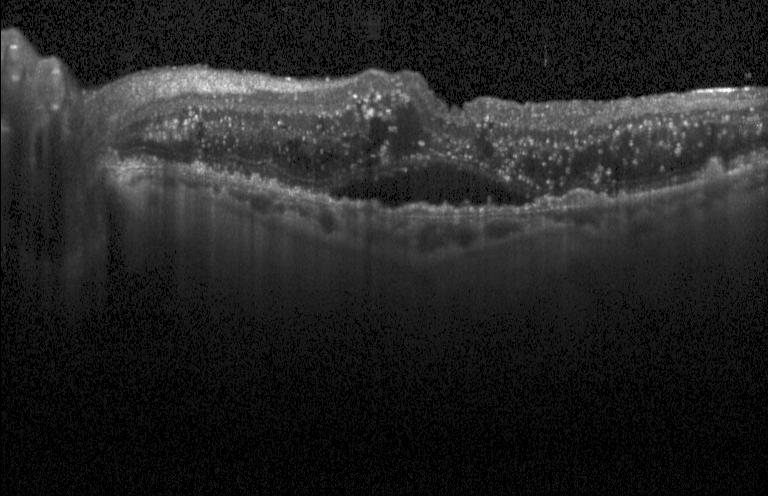

The scan shows CNV.